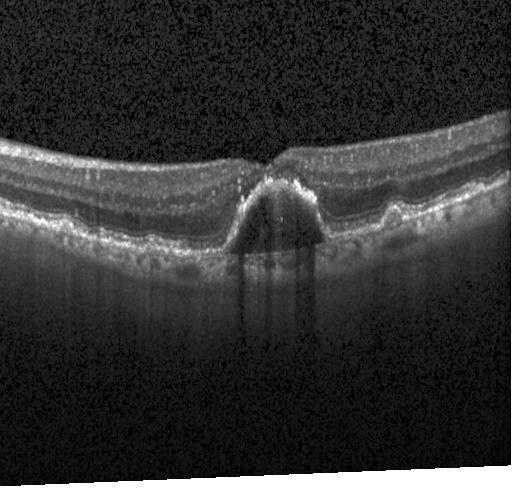
Diagnosis: a choroidal neovascular membrane.